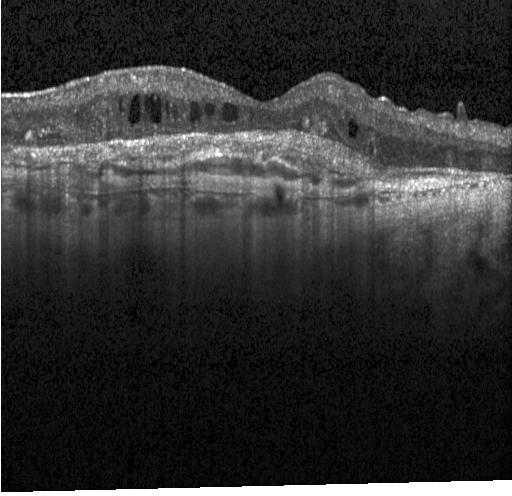 Fovea-centered. Spectral-domain OCT. Optical coherence tomography scan. Heidelberg Spectralis.
A choroidal neovascular membrane.